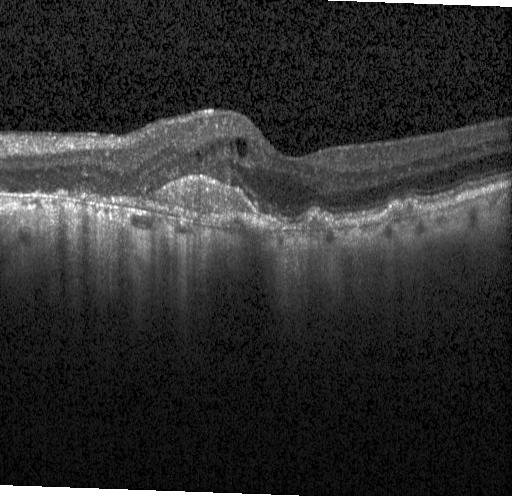

Instrument: Heidelberg Spectralis. OCT B-scan. Finding: a choroidal neovascular membrane.